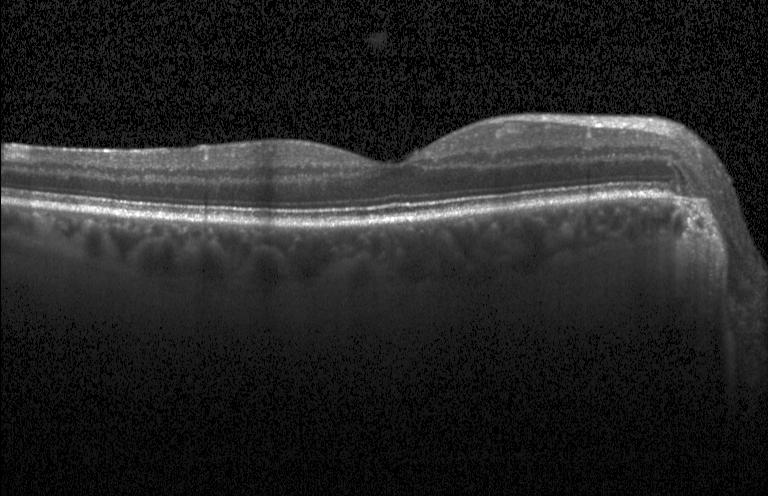 Impression: neither choroidal neovascularization, diabetic macular edema, nor drusen.